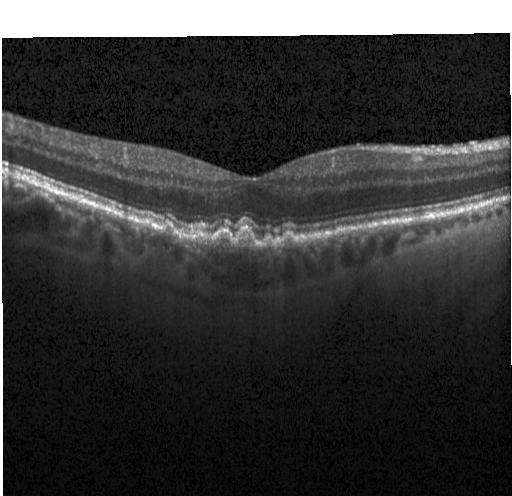

Retinal OCT cross-section. Spectral-domain OCT. The scan shows drusen.